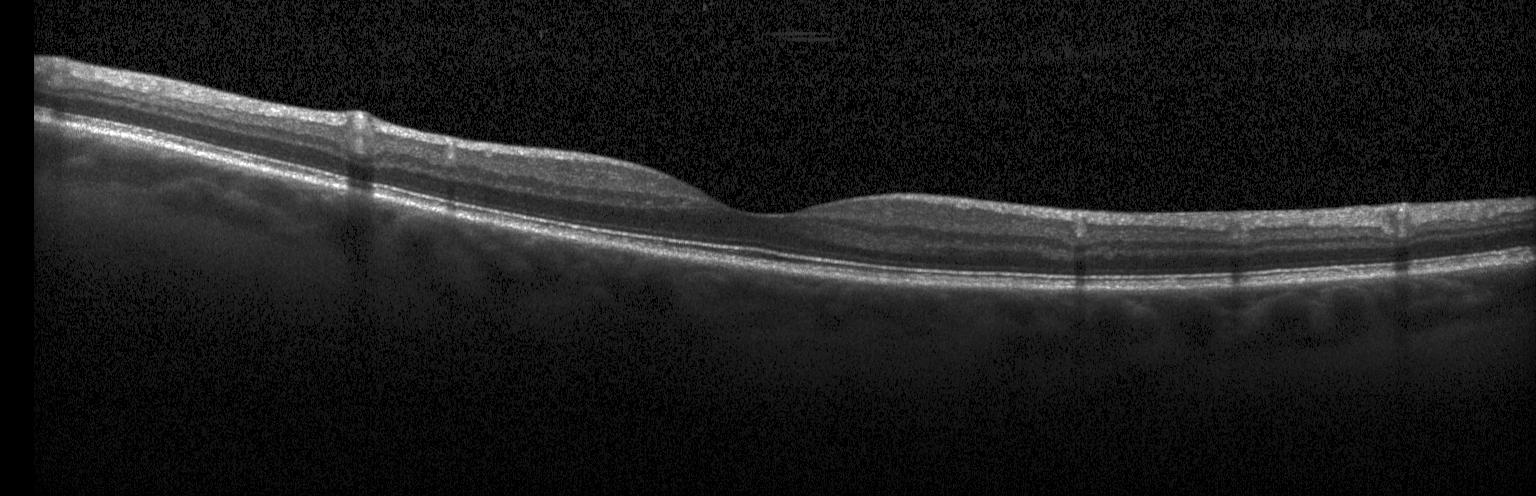
The scan shows no evidence of choroidal neovascularization, diabetic macular edema, or drusen.